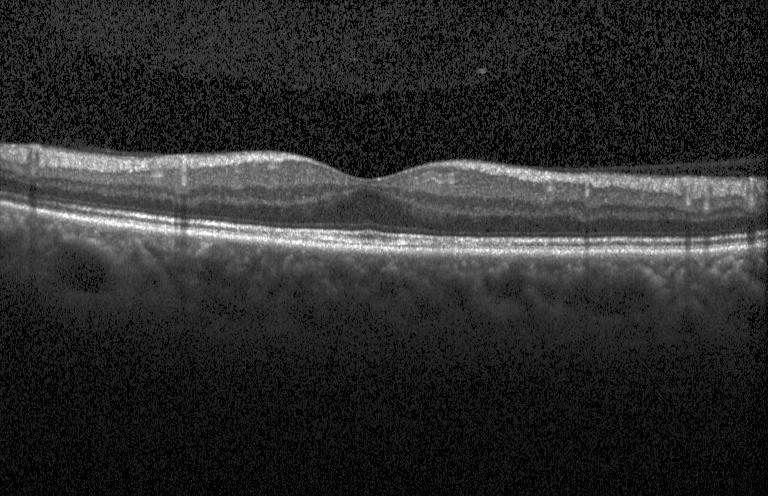 Diagnosis: neither CNV, DME, nor drusen.